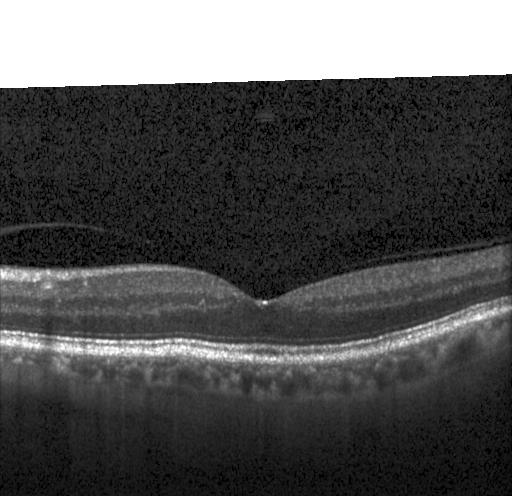 Assessment: neither choroidal neovascularization, diabetic macular edema, nor drusen.